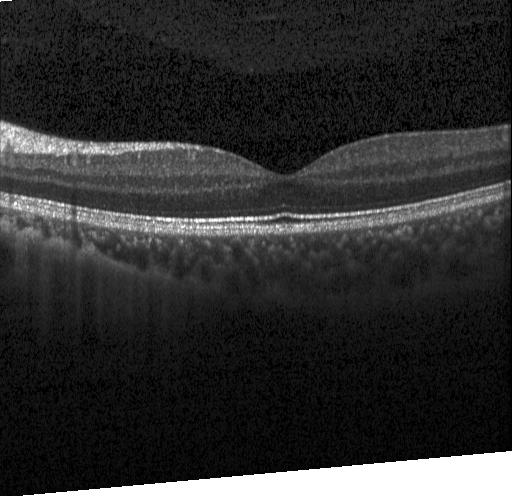 Spectral-domain OCT, macular scan, OCT line scan, instrument: Heidelberg Spectralis — OCT finding: no evidence of choroidal neovascularization, diabetic macular edema, or drusen.